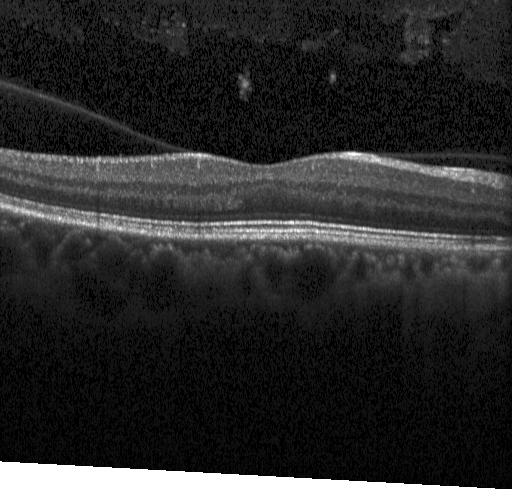

OCT finding: no CNV, no DME, and no drusen.